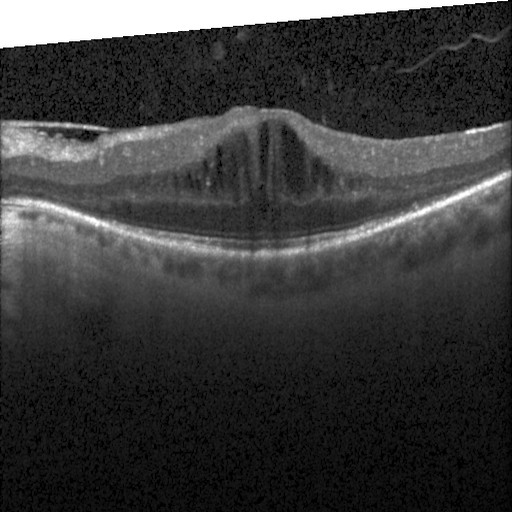
OCT B-scan
Diagnosis: diabetic macular edema.